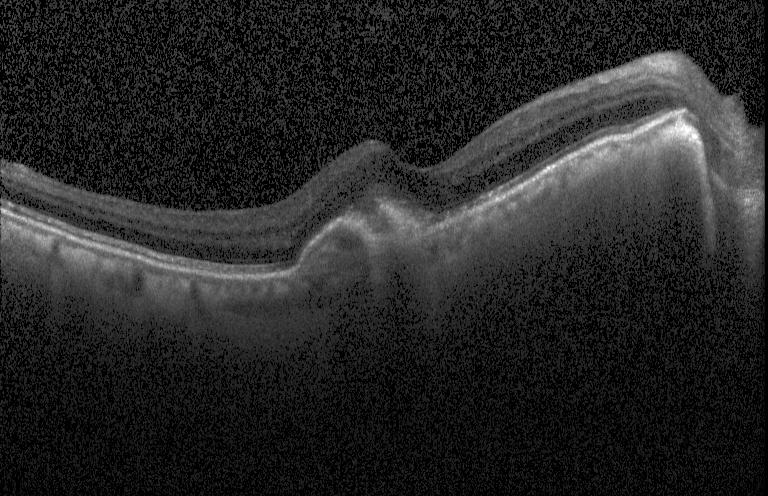
Acquired on a Heidelberg Spectralis · through the macula · retinal OCT cross-section.
A choroidal neovascular membrane.